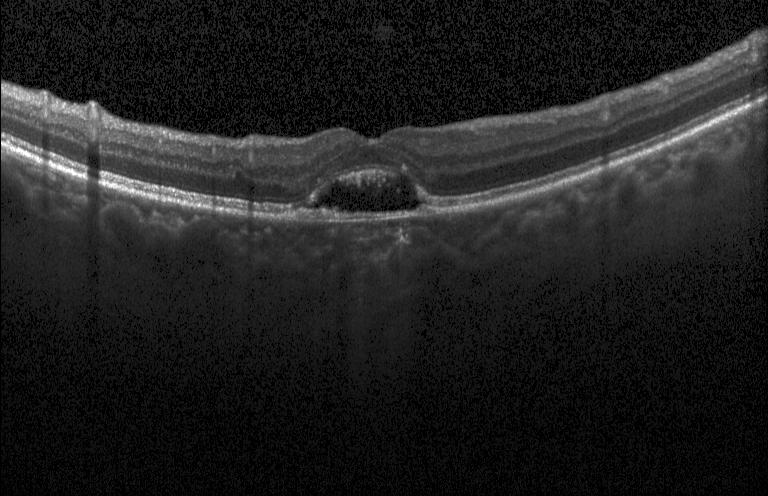 OCT B-scan; through the macula; spectral-domain OCT
Finding: CNV.